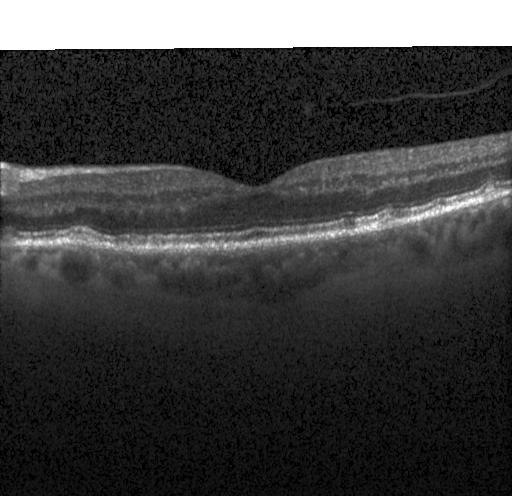

Optical coherence tomography scan. Heidelberg Spectralis. Sub-RPE drusenoid deposits.